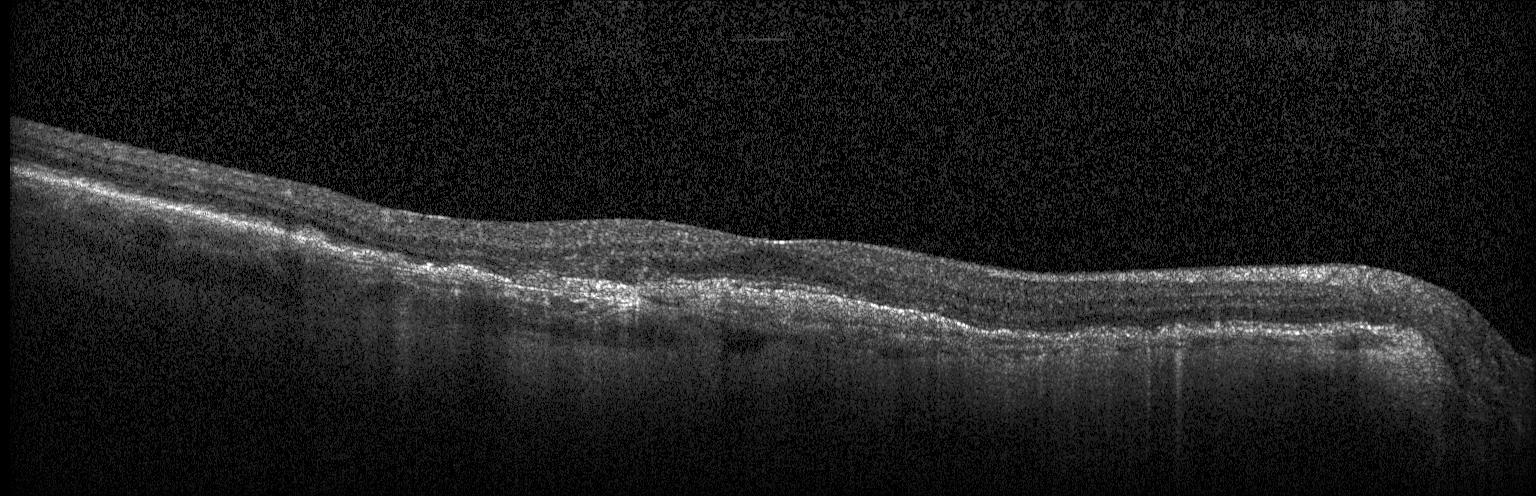

OCT line scan.
Assessment: a choroidal neovascular membrane.